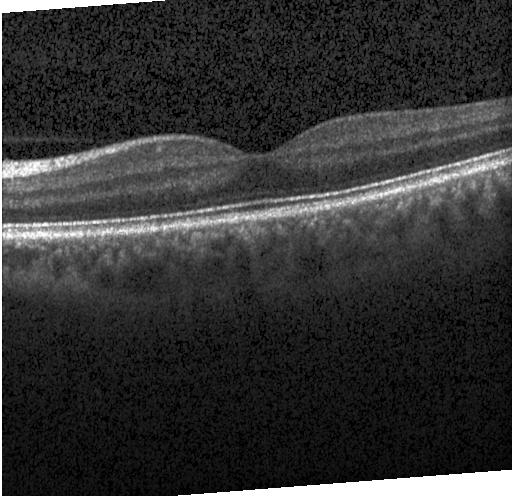
Optical coherence tomography B-scan
Diagnosis: no CNV, no DME, and no drusen.